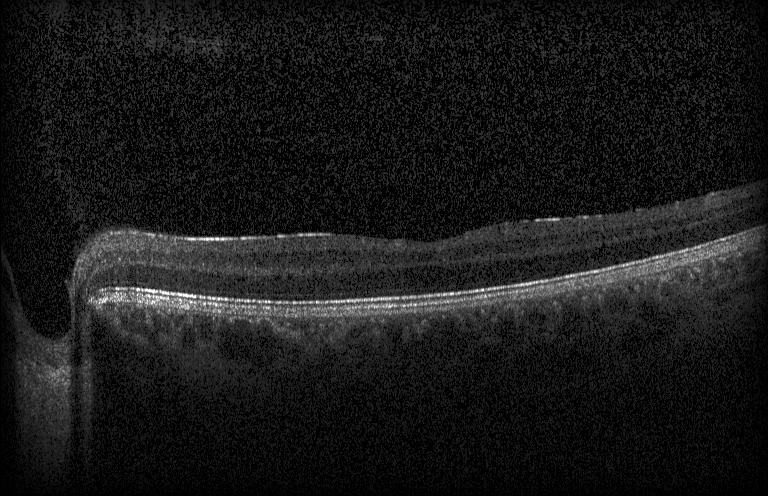
Macular OCT: no choroidal neovascularization, diabetic macular edema, or drusen.